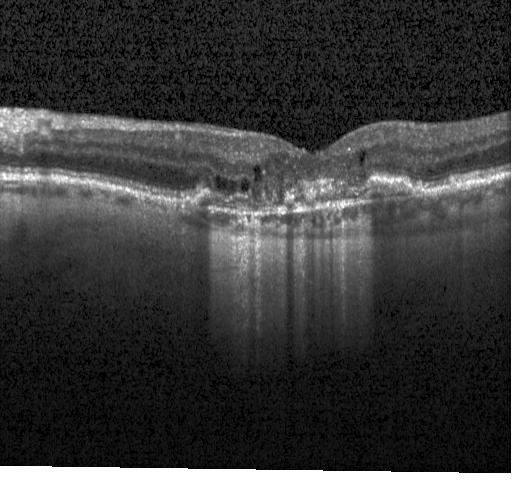
Retinal OCT cross-section — A choroidal neovascular membrane.